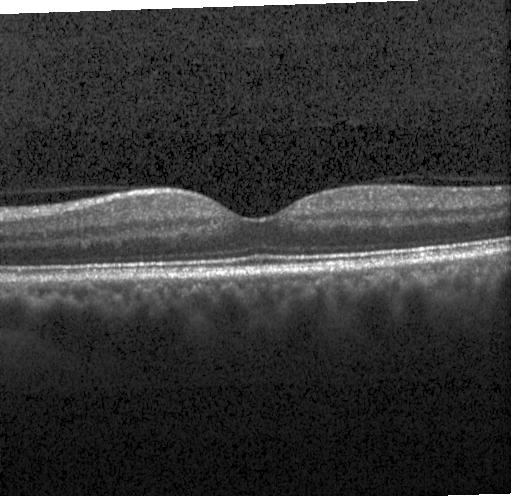

Macular scan · Heidelberg Spectralis · OCT line scan
OCT finding: no choroidal neovascularization, diabetic macular edema, or drusen.